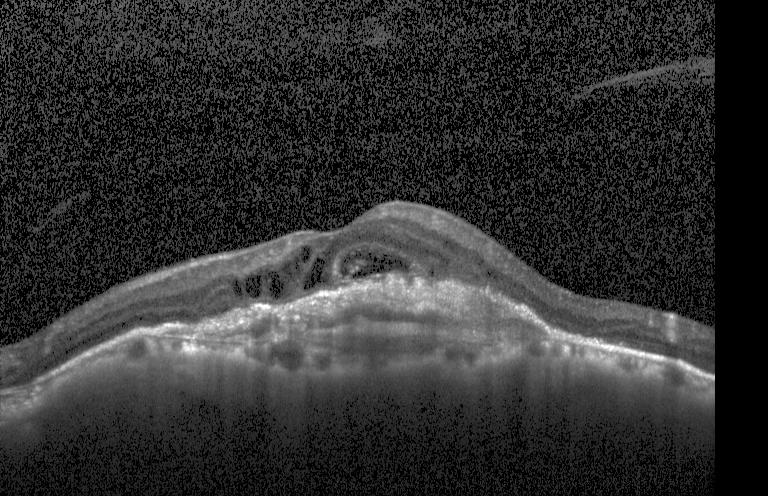

Macular scan, optical coherence tomography B-scan, instrument: Heidelberg Spectralis — Impression: choroidal neovascularization.